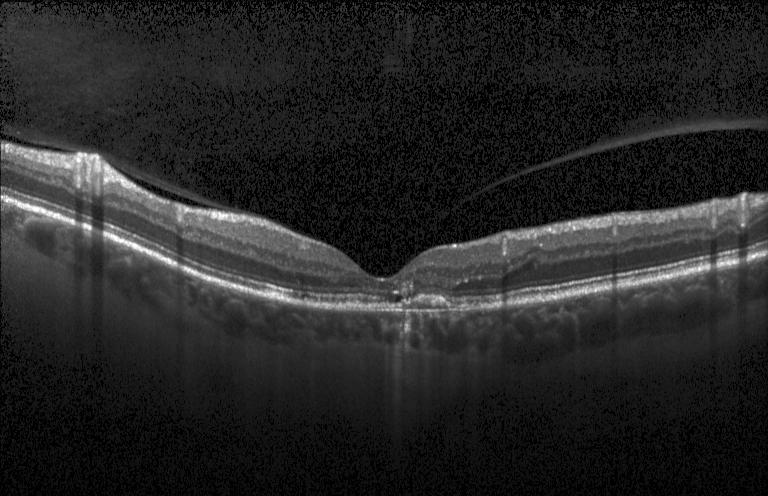
Fovea-centered, SD-OCT, Heidelberg Spectralis, OCT B-scan — Diagnosis: choroidal neovascularization.